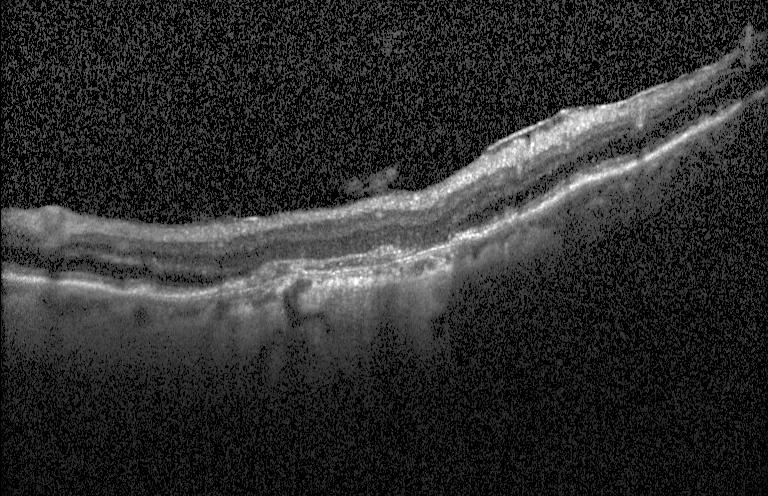
OCT B-scan.
Macular OCT: a choroidal neovascular membrane.